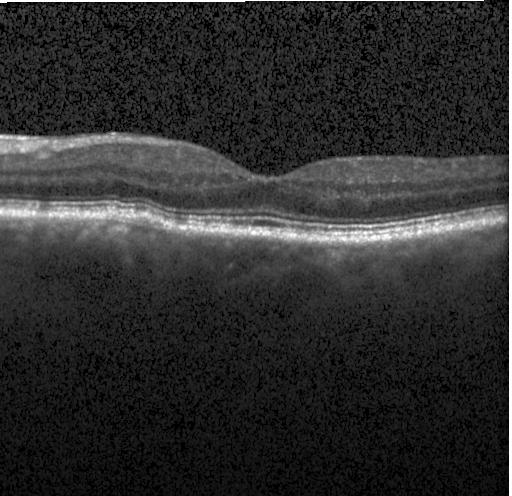

Retinal OCT B-scan
Impression: sub-RPE drusenoid deposits.